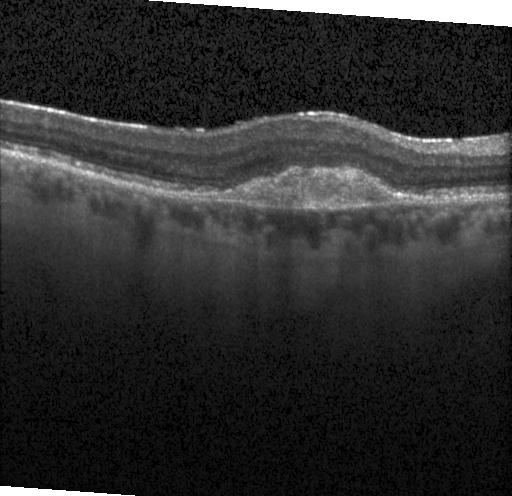

Spectral-domain OCT B-scan: choroidal neovascularization.